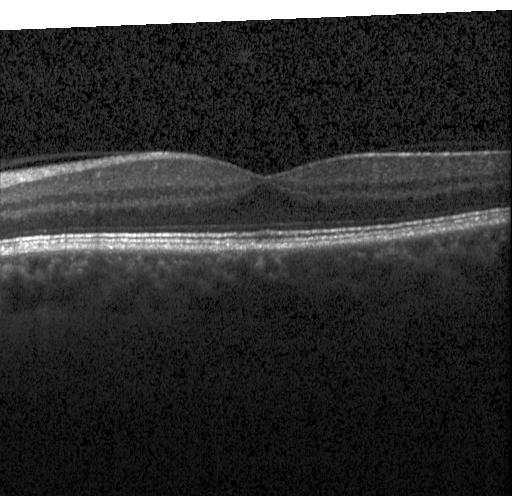
This B-scan demonstrates no CNV, DME, or drusen.